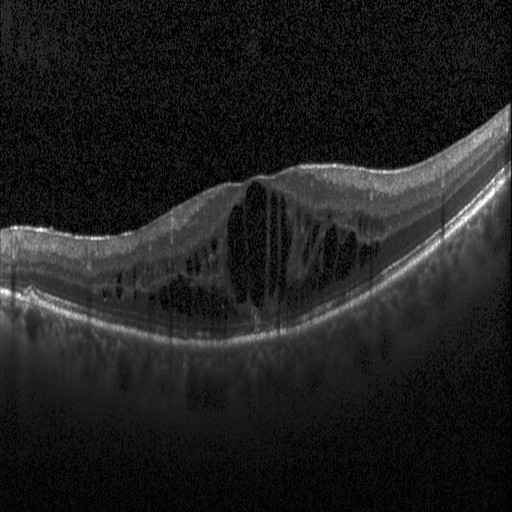 Spectral-domain OCT B-scan: DME.